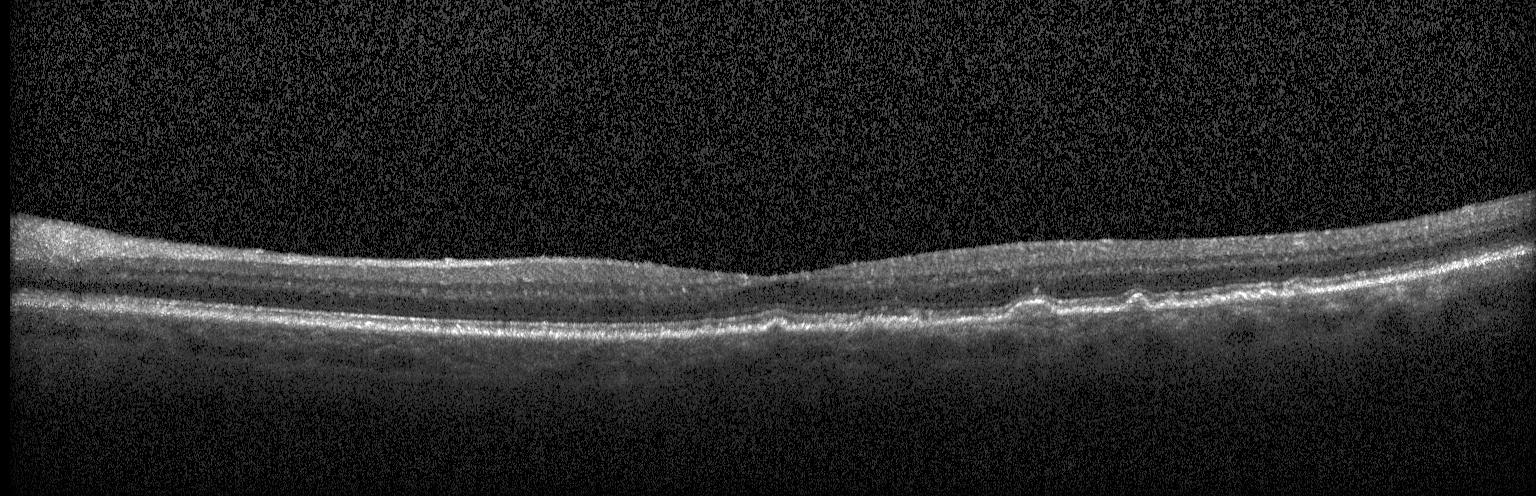
Retinal OCT B-scan
Sub-RPE drusenoid deposits.